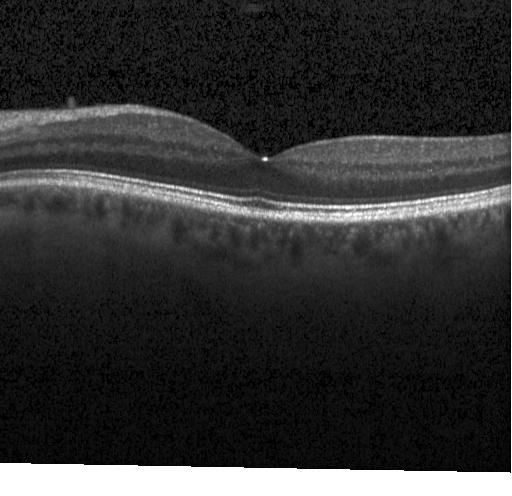 Finding: neither choroidal neovascularization, diabetic macular edema, nor drusen.